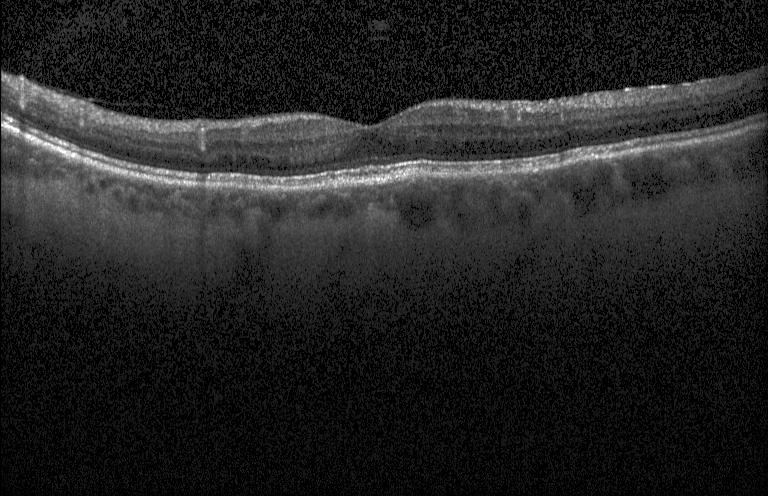

Macular OCT: no CNV, DME, or drusen.